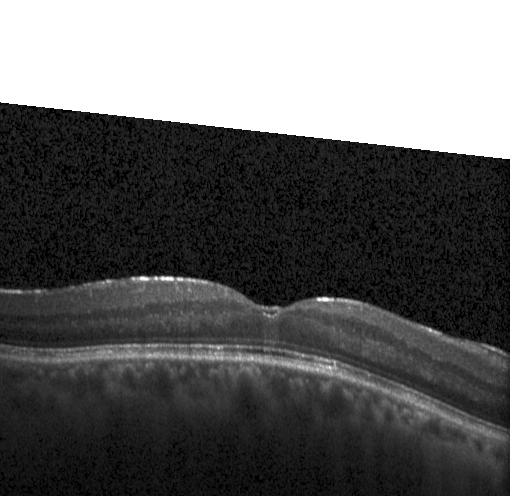
Finding: no CNV, no DME, and no drusen.